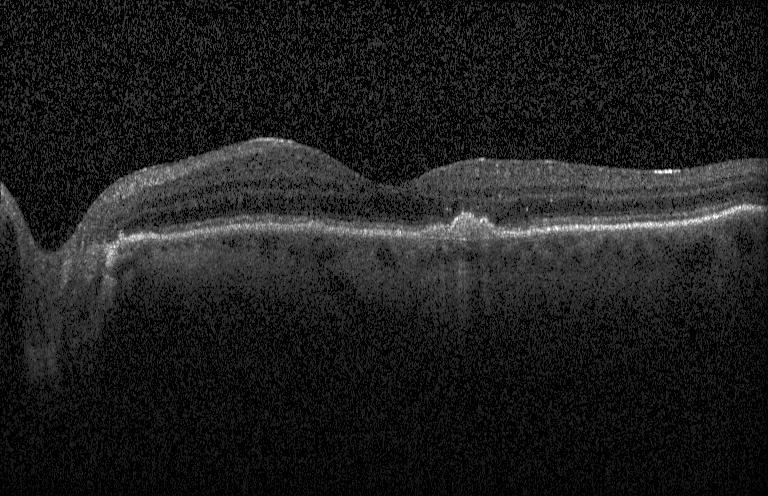
Optical coherence tomography B-scan; macular scan; spectral-domain optical coherence tomography; Heidelberg Spectralis OCT system — Impression: multiple drusen.